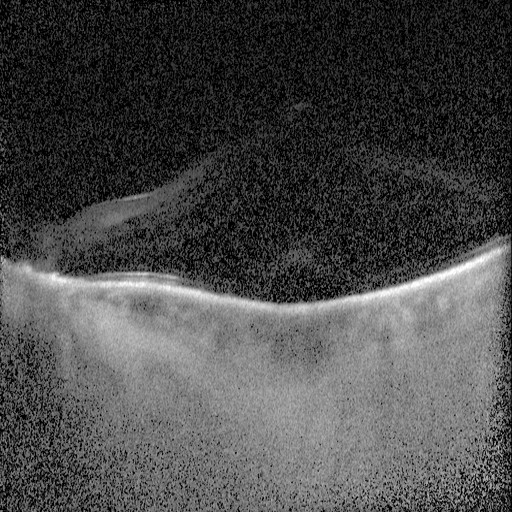 Fovea-centered, SD-OCT, OCT line scan — OCT finding: diabetic macular edema.